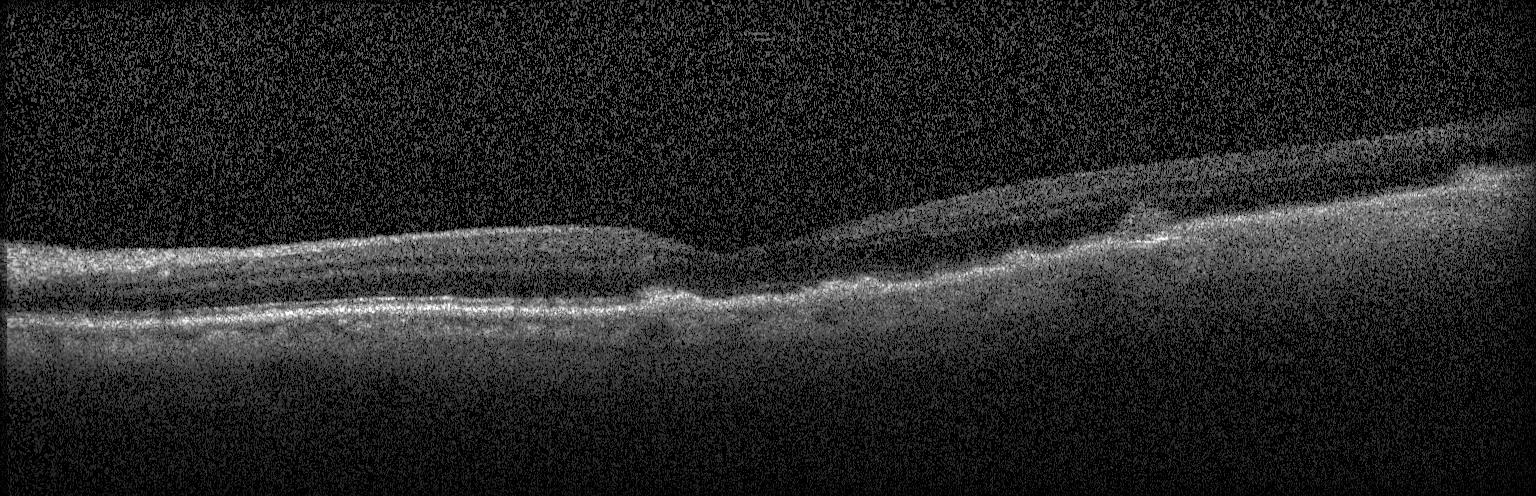 OCT line scan. Centered on the fovea. Acquired on a Heidelberg Spectralis.
Finding: choroidal neovascularization (CNV).